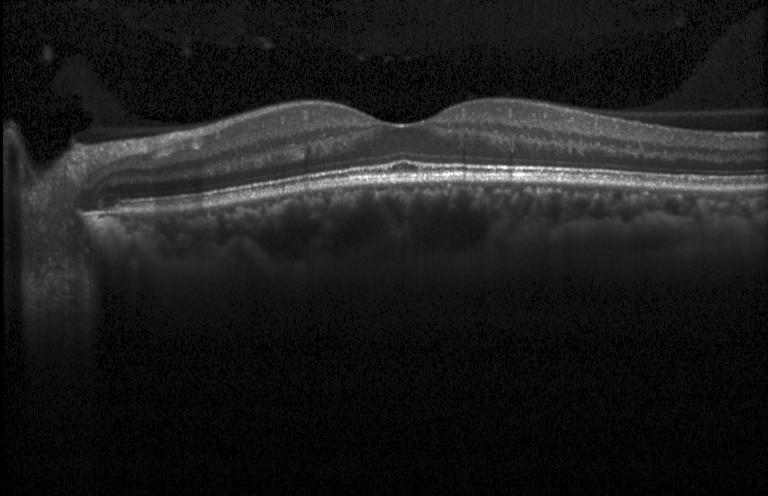
OCT B-scan; macular scan; acquired on a Heidelberg Spectralis
Impression: no choroidal neovascularization, no diabetic macular edema, and no drusen.